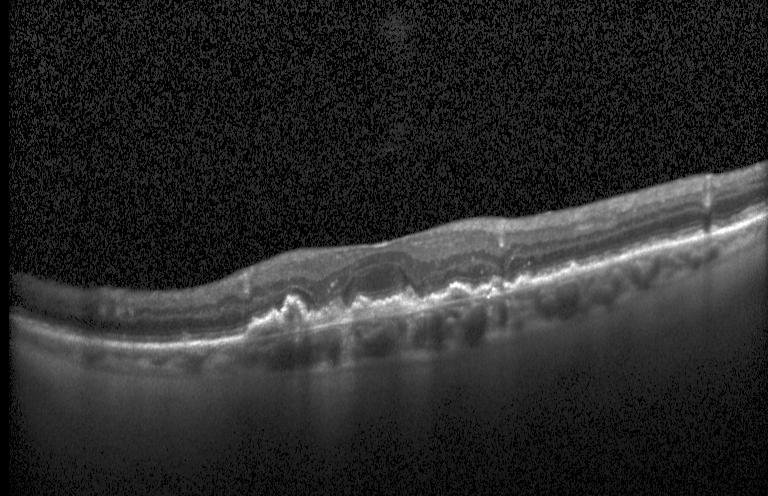
Retinal OCT B-scan, Heidelberg Spectralis OCT system. Diagnosis: CNV.